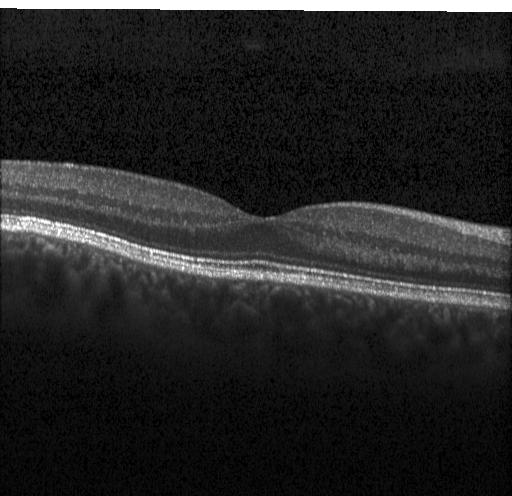

Spectral-domain OCT B-scan: no choroidal neovascularization, diabetic macular edema, or drusen.